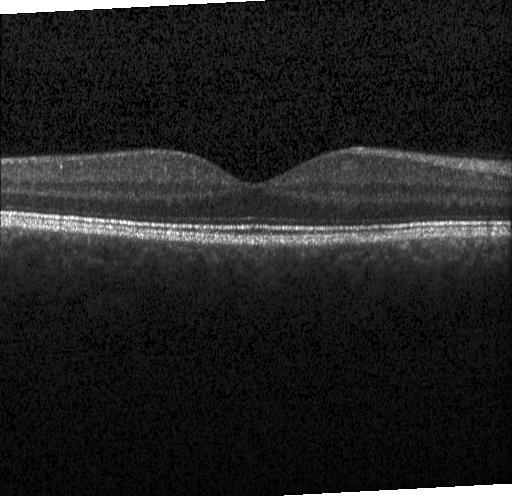
Acquired on a Heidelberg Spectralis, retinal OCT cross-section.
Macular OCT: neither choroidal neovascularization, diabetic macular edema, nor drusen.